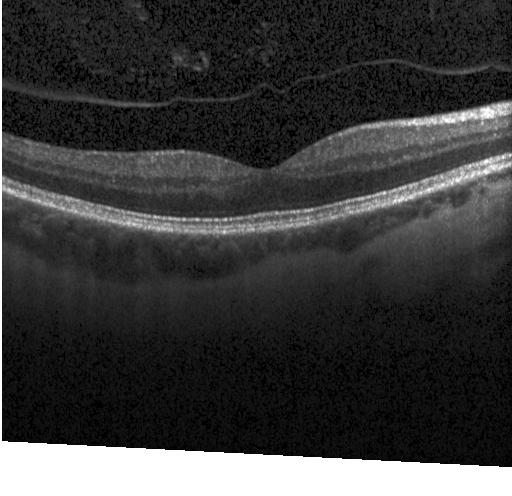

OCT line scan; instrument: Heidelberg Spectralis. Impression: no evidence of choroidal neovascularization, diabetic macular edema, or drusen.